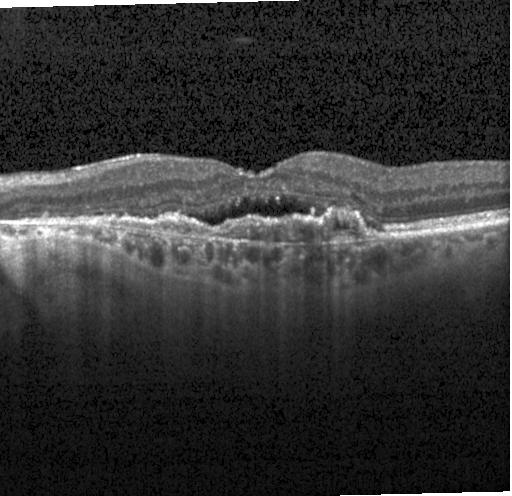 Optical coherence tomography B-scan
Impression: a choroidal neovascular membrane.